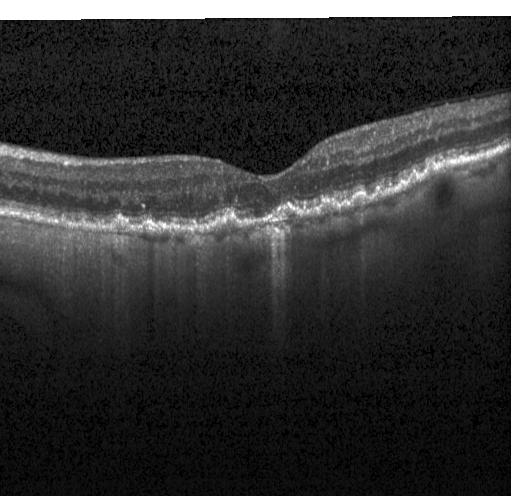 Heidelberg Spectralis OCT system; OCT line scan.
Diagnosis: drusen.